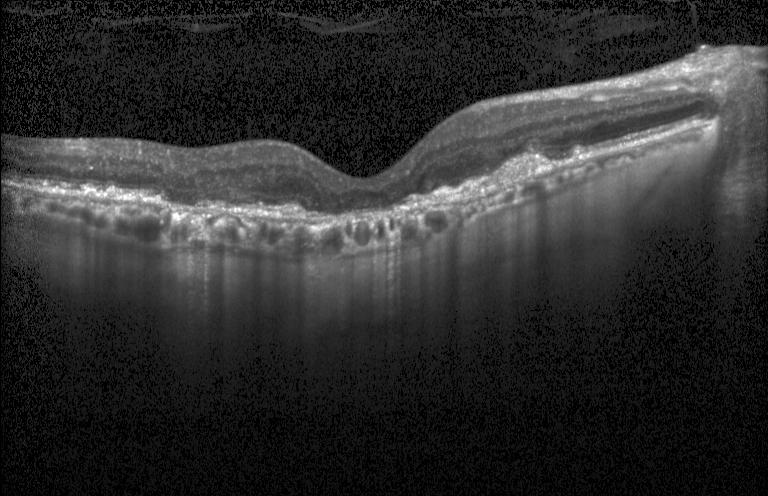
Macular scan, OCT B-scan, spectral-domain optical coherence tomography
Impression: a choroidal neovascular membrane.